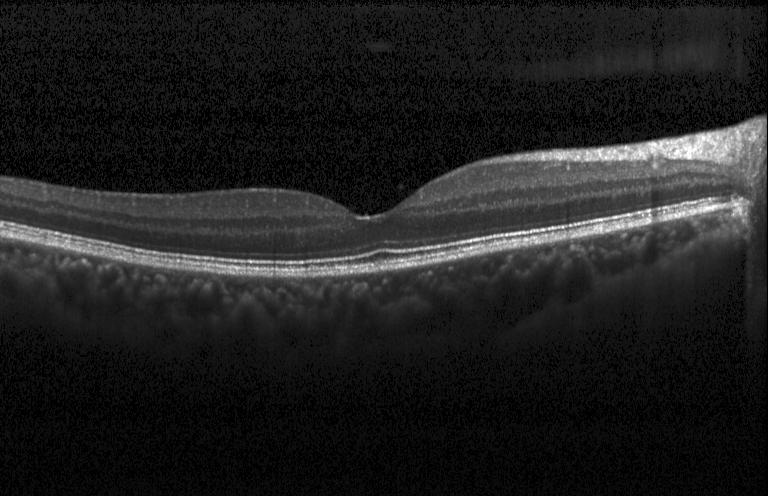

SD-OCT. Optical coherence tomography scan
Diagnosis: no CNV, DME, or drusen.